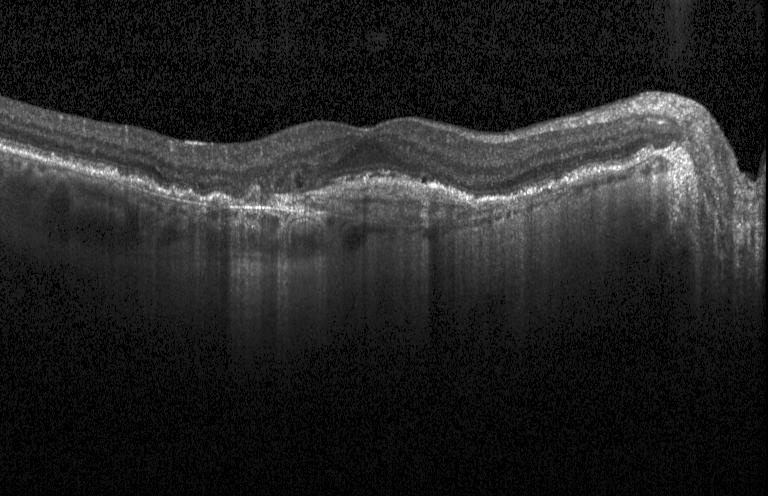
OCT B-scan. Spectral-domain optical coherence tomography. Finding: choroidal neovascularization (CNV).